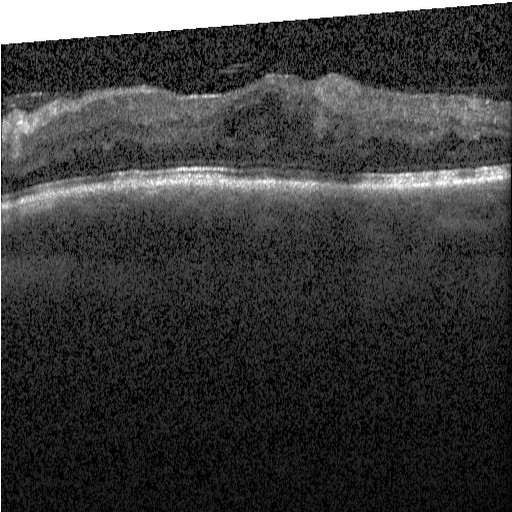
Optical coherence tomography B-scan.
Finding: diabetic macular edema.